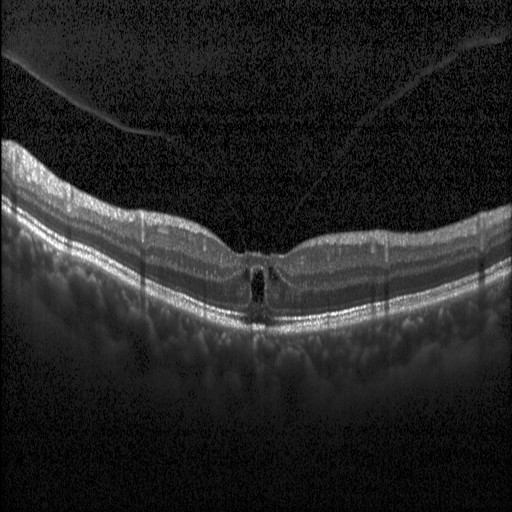 Dx: diabetic macular edema.